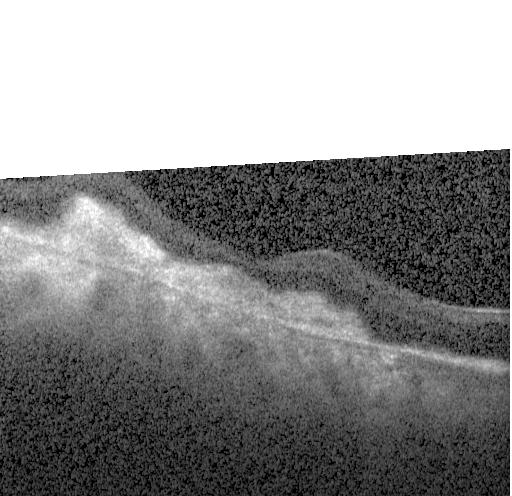

Instrument: Heidelberg Spectralis · retinal OCT B-scan
OCT finding: choroidal neovascularization (CNV).